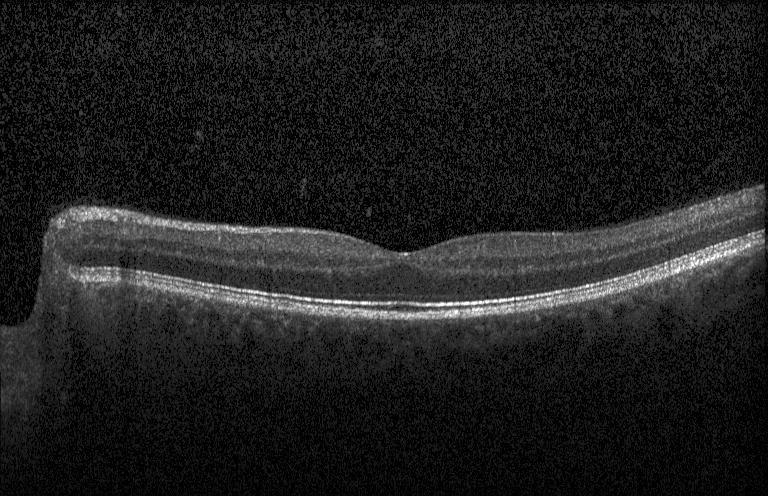
Macular OCT demonstrating neither choroidal neovascularization, diabetic macular edema, nor drusen.